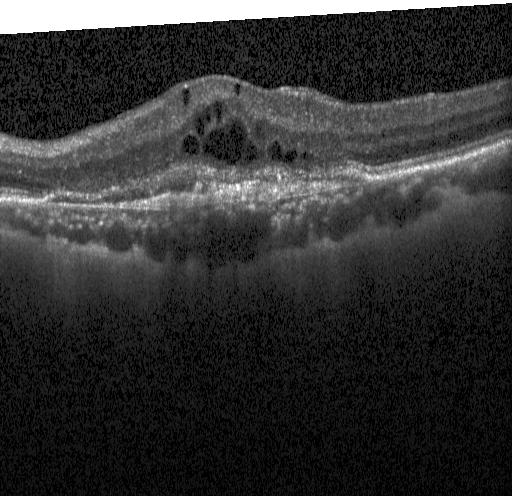 Spectral-domain OCT B-scan: choroidal neovascularization (CNV).